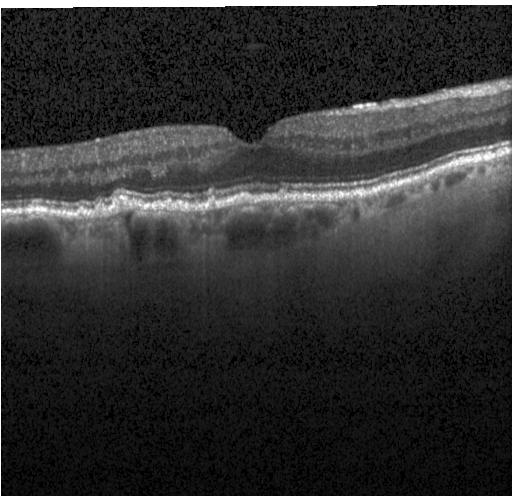

Finding: sub-RPE drusenoid deposits.